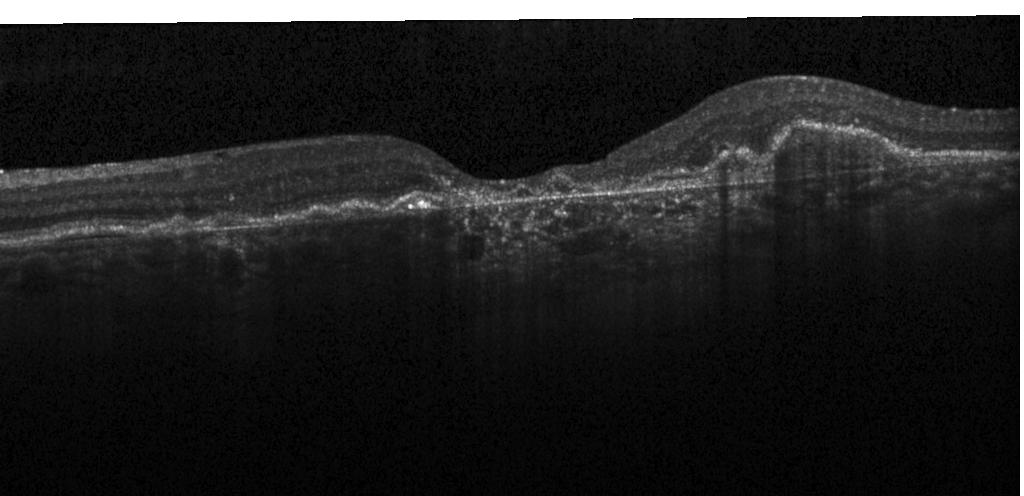 CNV.